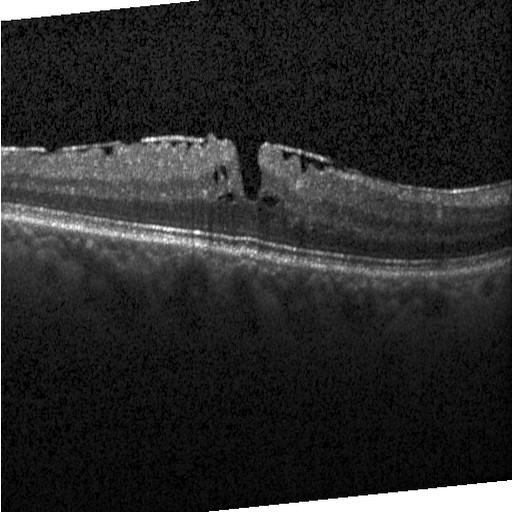

Heidelberg Spectralis OCT system, OCT B-scan, SD-OCT. Dx: DME.